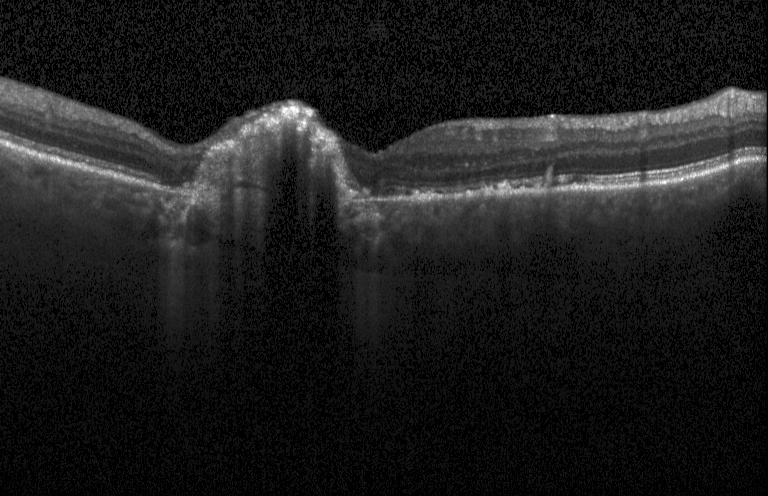 Centered on the fovea. OCT line scan. This B-scan demonstrates choroidal neovascularization (CNV).